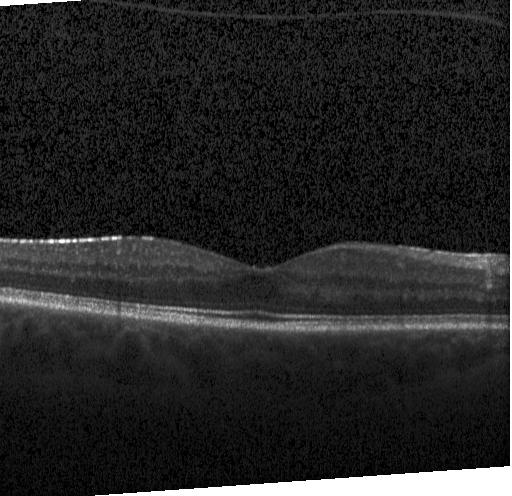 OCT finding: no choroidal neovascularization, diabetic macular edema, or drusen.